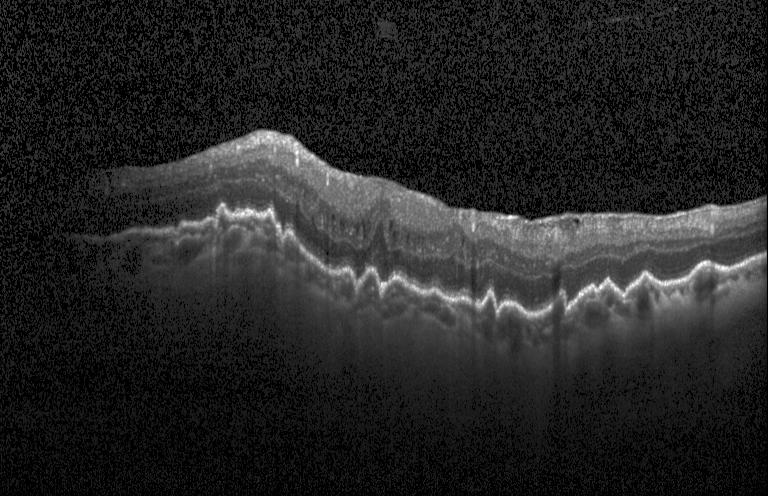

Acquired on a Heidelberg Spectralis; retinal OCT cross-section. Impression: CNV.